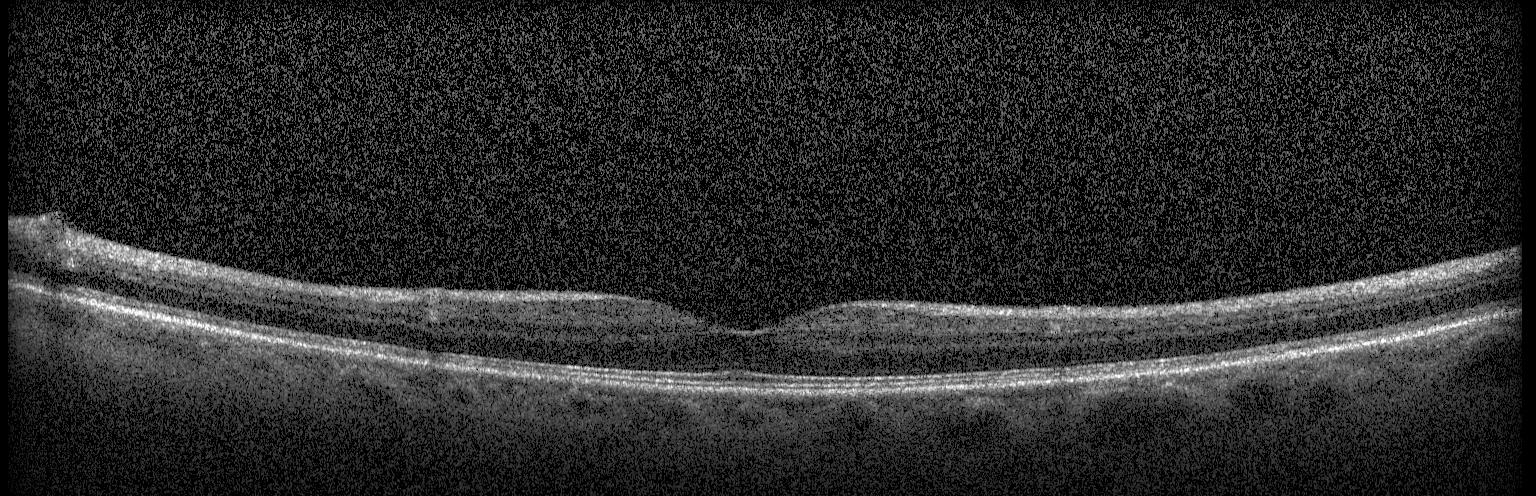

Optical coherence tomography B-scan. Heidelberg Spectralis.
OCT finding: neither CNV, DME, nor drusen.